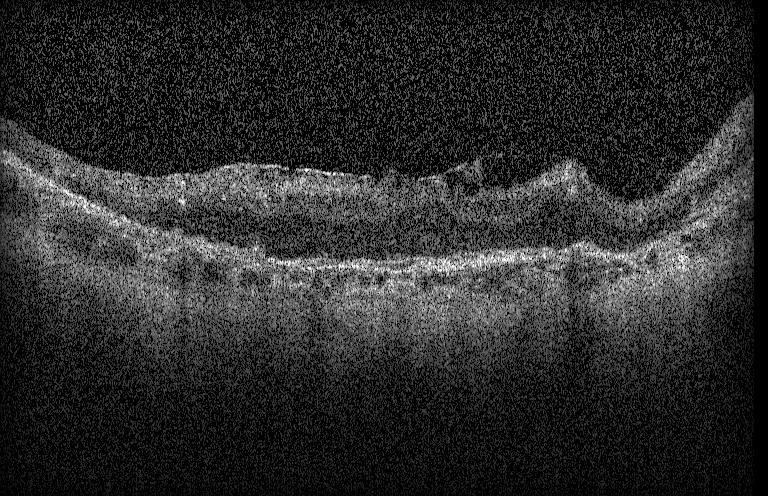
Retinal OCT cross-section — Assessment: a choroidal neovascular membrane.